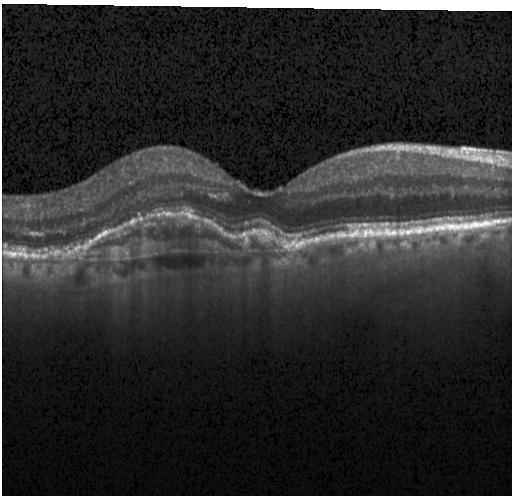 Retinal OCT cross-section · centered on the fovea.
The scan shows a choroidal neovascular membrane.